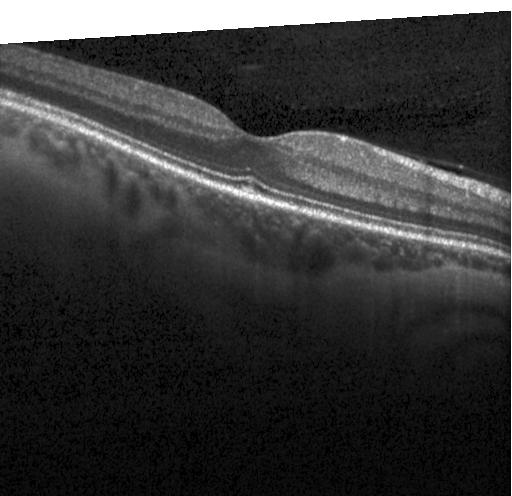 Finding: no choroidal neovascularization, diabetic macular edema, or drusen.